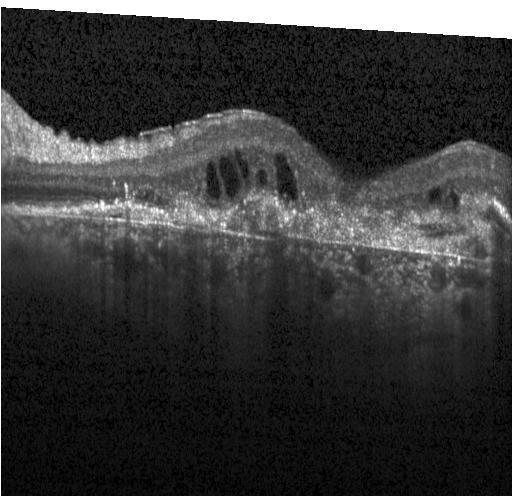

Retinal OCT cross-section showing a choroidal neovascular membrane.